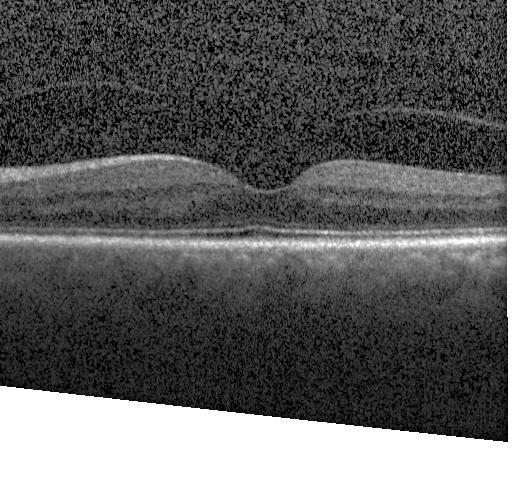 Optical coherence tomography B-scan · acquired on a Heidelberg Spectralis · spectral-domain optical coherence tomography · centered on the fovea. OCT finding: no CNV, DME, or drusen.